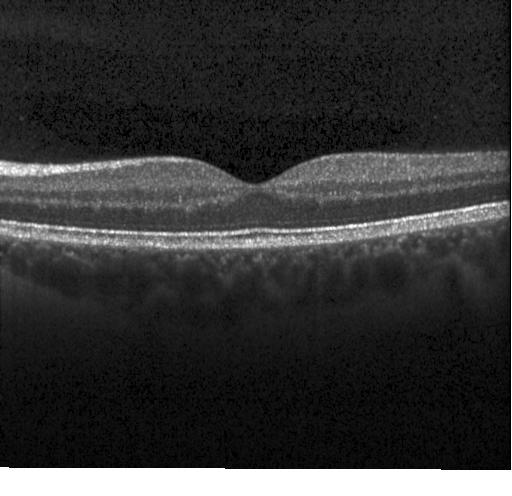
Finding: neither choroidal neovascularization, diabetic macular edema, nor drusen.